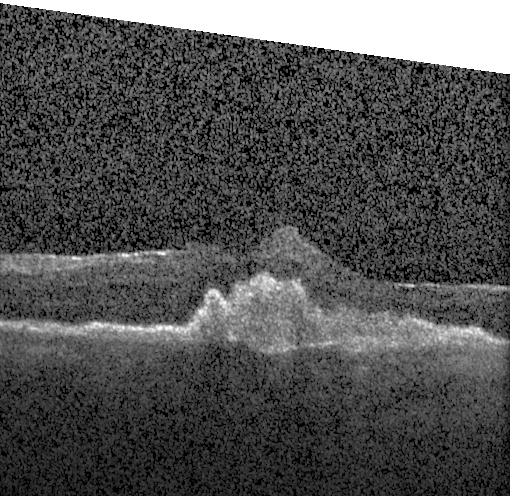
Dx: a choroidal neovascular membrane.